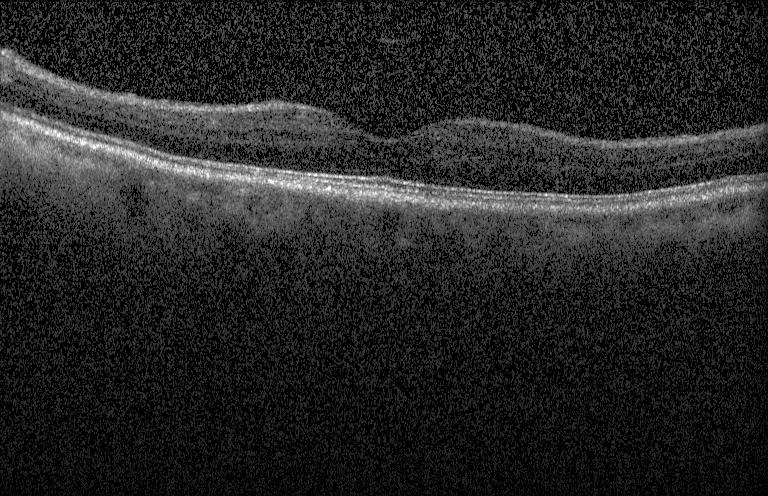

Instrument: Heidelberg Spectralis, OCT B-scan — Neither CNV, DME, nor drusen.